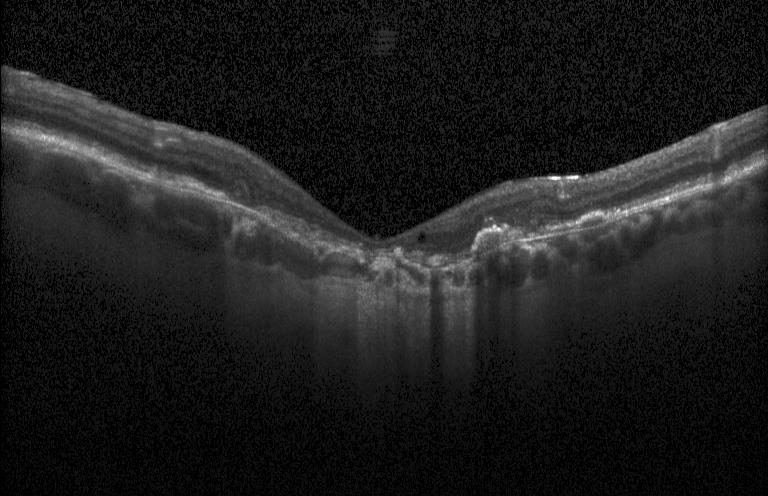 Retinal OCT B-scan; centered on the fovea. Impression: CNV.